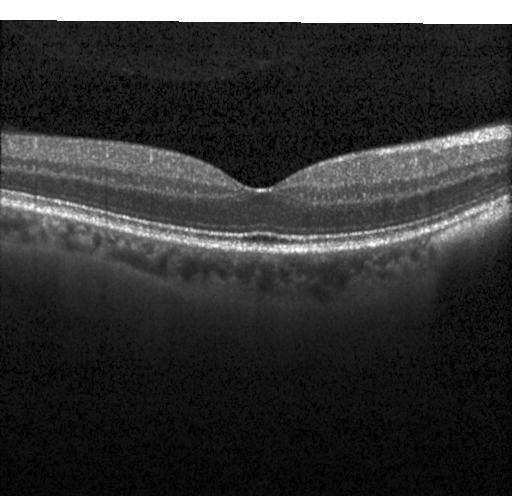
Spectral-domain optical coherence tomography, through the macula, optical coherence tomography scan — Diagnosis: no CNV, DME, or drusen.